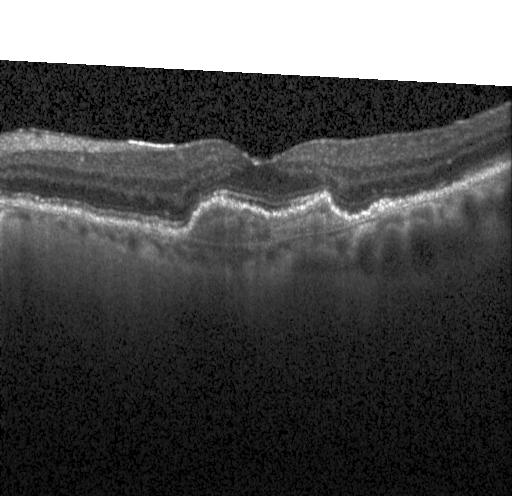

Macular OCT: a choroidal neovascular membrane.